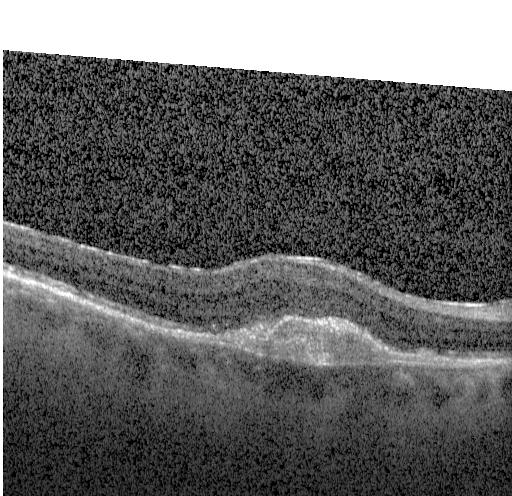
Spectral-domain OCT. Acquired on a Heidelberg Spectralis. OCT line scan. Centered on the fovea. This B-scan demonstrates choroidal neovascularization (CNV).